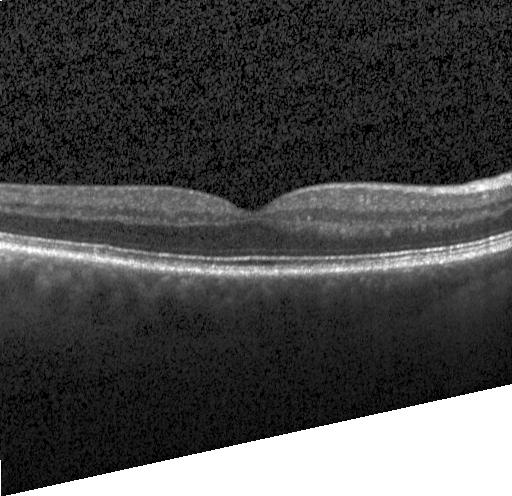
No choroidal neovascularization, diabetic macular edema, or drusen.